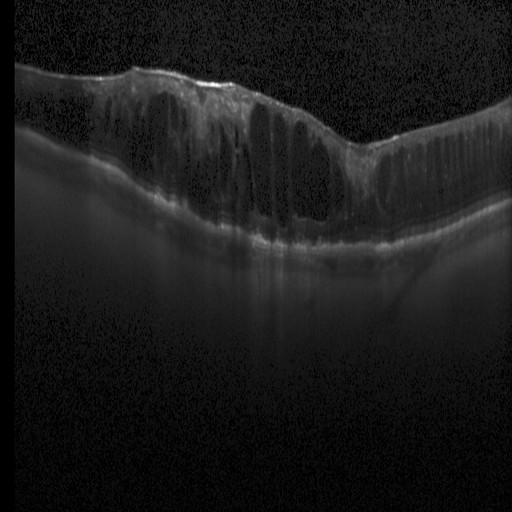
OCT line scan · spectral-domain OCT — Diabetic macular edema.